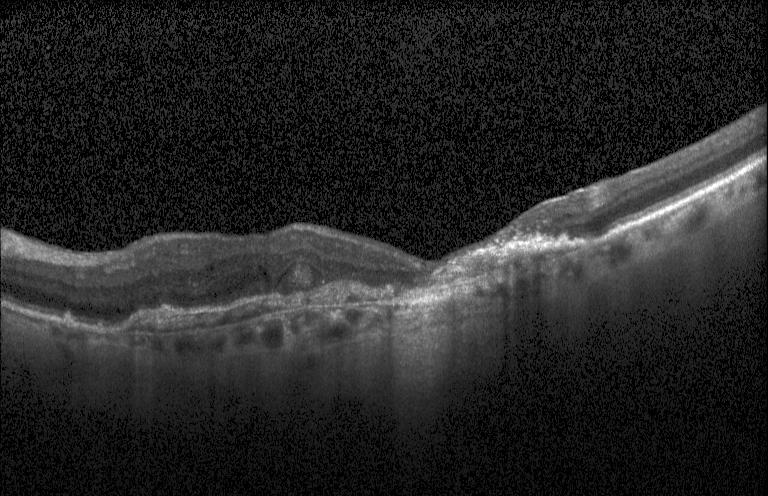 OCT B-scan showing choroidal neovascularization (CNV).